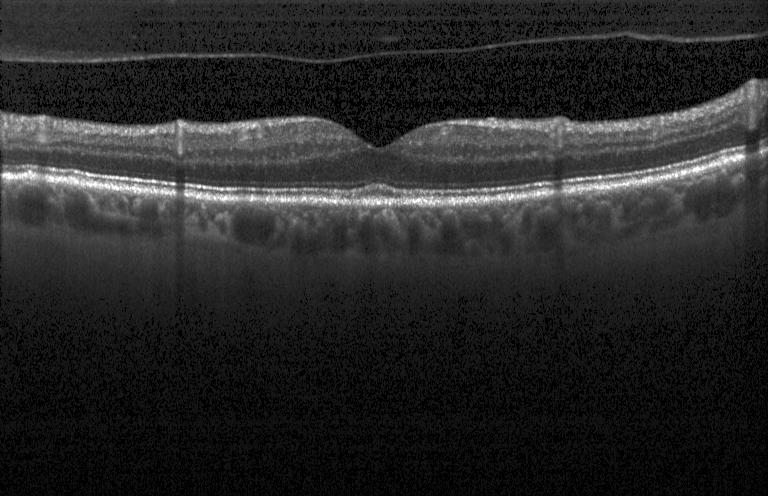
Diagnosis: no evidence of choroidal neovascularization, diabetic macular edema, or drusen.